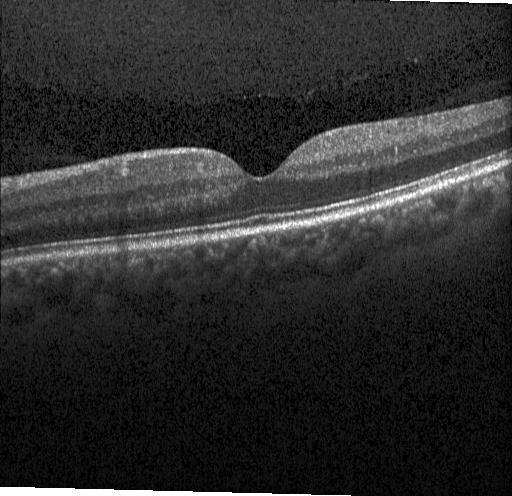
Acquired on a Heidelberg Spectralis. Optical coherence tomography B-scan. SD-OCT.
Impression: no choroidal neovascularization, diabetic macular edema, or drusen.